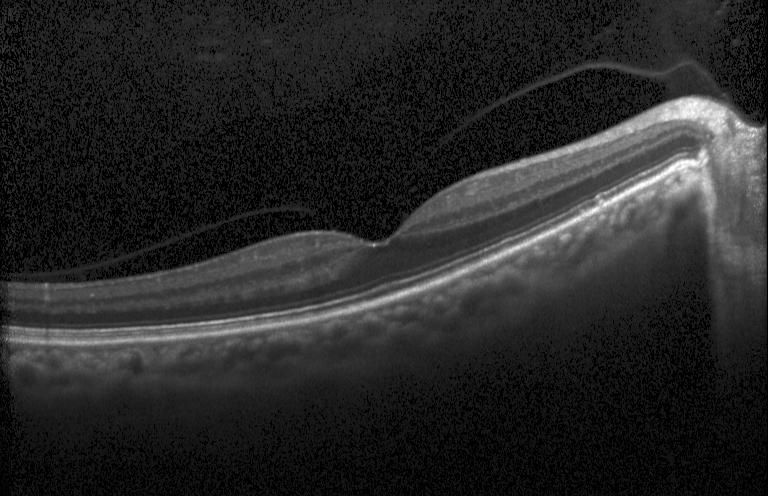
OCT scan showing no choroidal neovascularization, diabetic macular edema, or drusen.